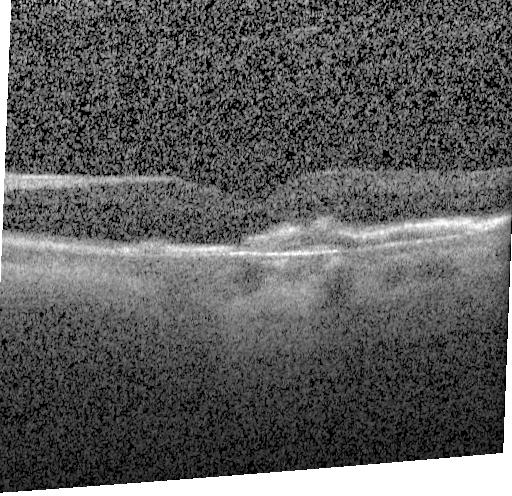
Retinal OCT cross-section
Diagnosis: a choroidal neovascular membrane.